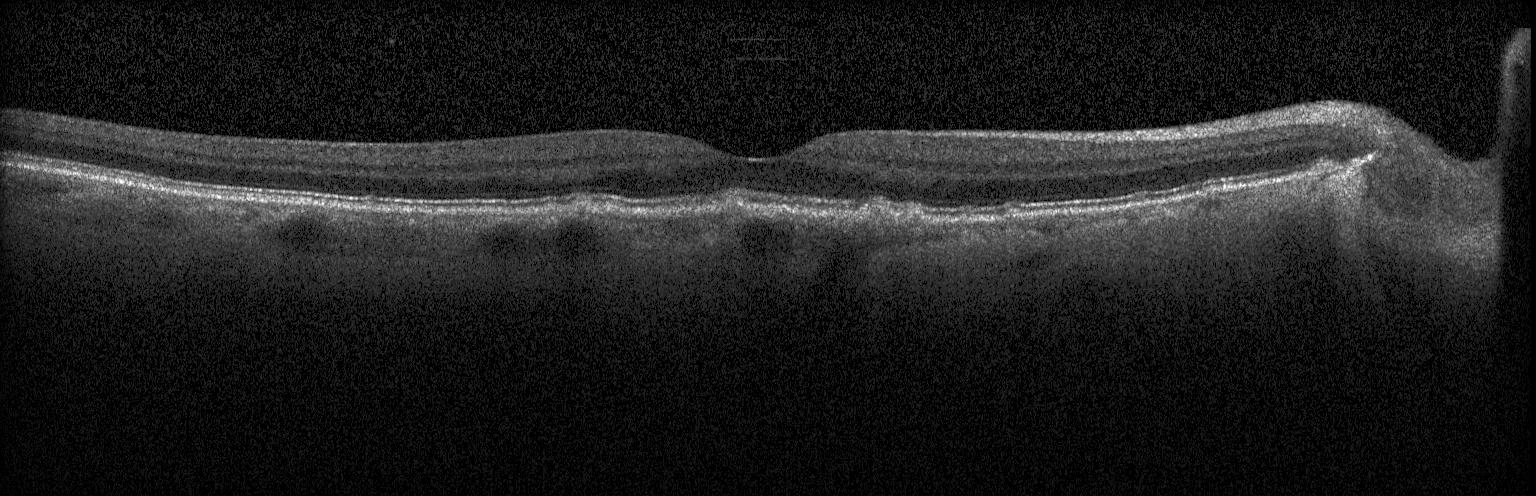

Finding: sub-RPE drusenoid deposits.